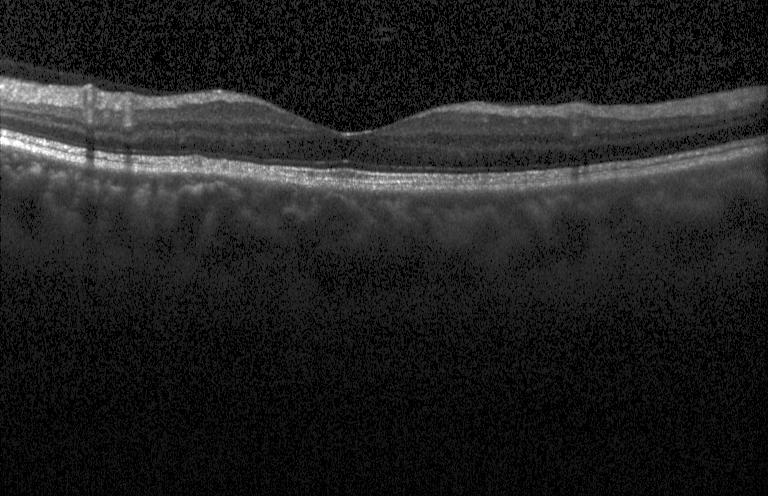
Heidelberg Spectralis OCT system. OCT line scan. Assessment: no choroidal neovascularization, no diabetic macular edema, and no drusen.